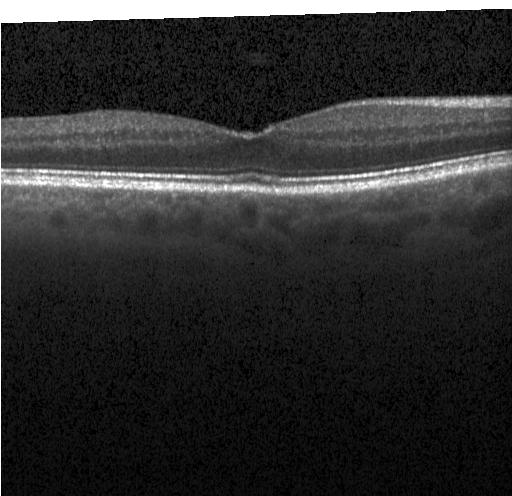
Optical coherence tomography scan
Diagnosis: no evidence of CNV, DME, or drusen.